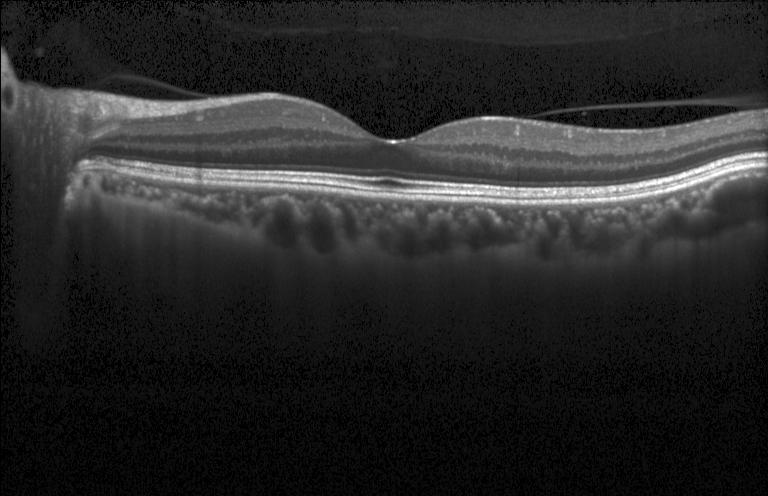 Diagnosis: no CNV, DME, or drusen.